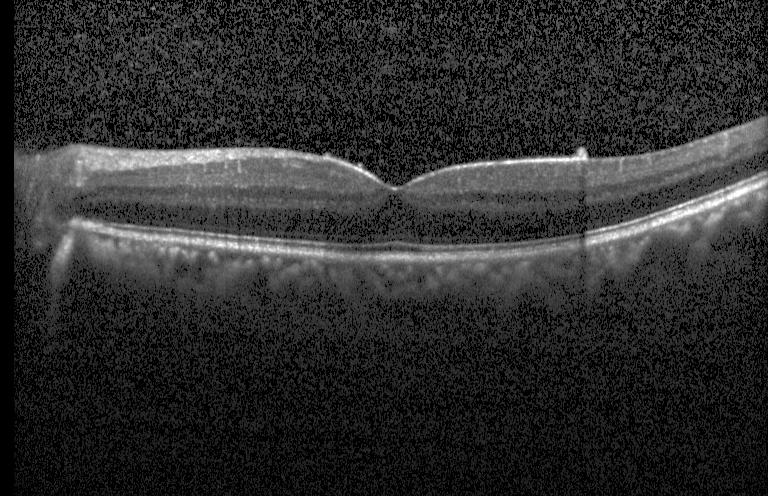 Assessment: neither choroidal neovascularization, diabetic macular edema, nor drusen.